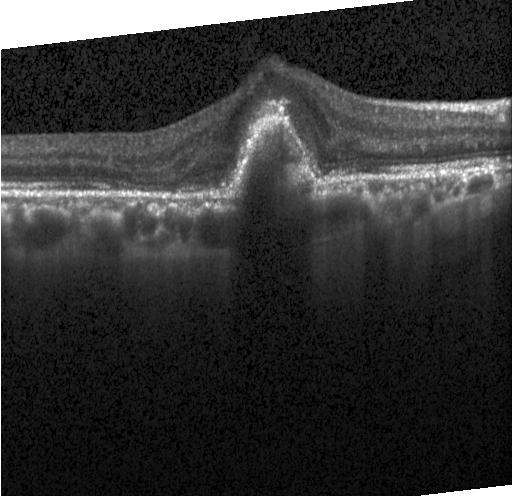

Spectral-domain optical coherence tomography · acquired on a Heidelberg Spectralis · optical coherence tomography scan — Impression: choroidal neovascularization (CNV).